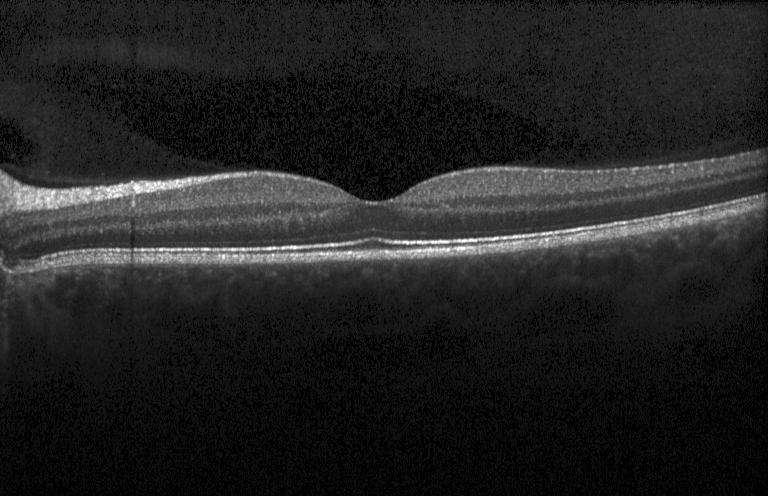

Optical coherence tomography B-scan — No choroidal neovascularization, no diabetic macular edema, and no drusen.